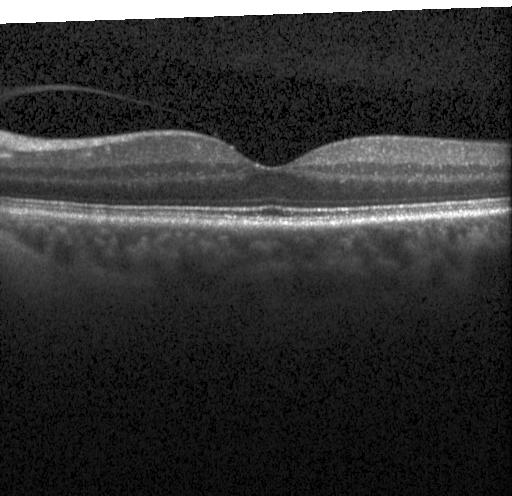
Retinal OCT cross-section; spectral-domain OCT
Diagnosis: no choroidal neovascularization, no diabetic macular edema, and no drusen.